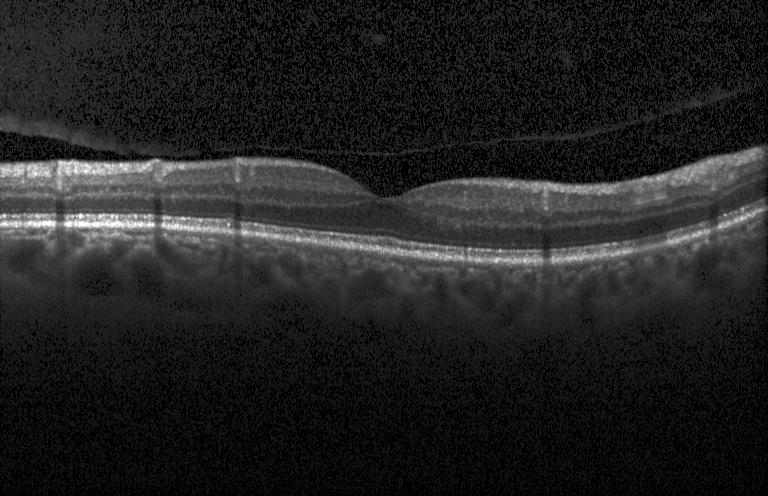
Finding: no CNV, DME, or drusen.